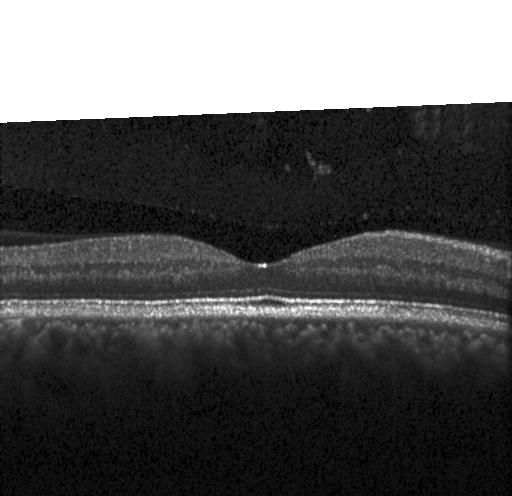

Through the macula. OCT line scan
OCT finding: no choroidal neovascularization, no diabetic macular edema, and no drusen.